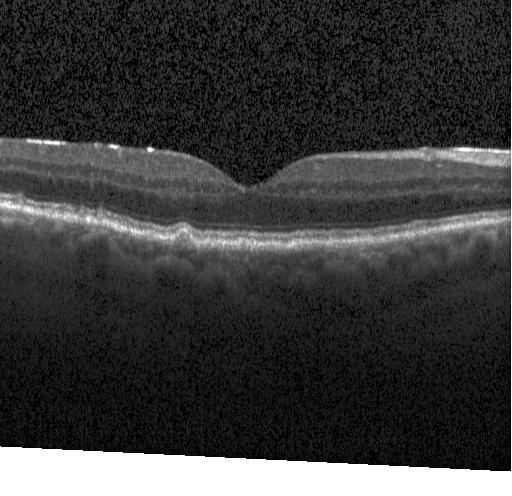 Diagnosis: sub-RPE drusenoid deposits.